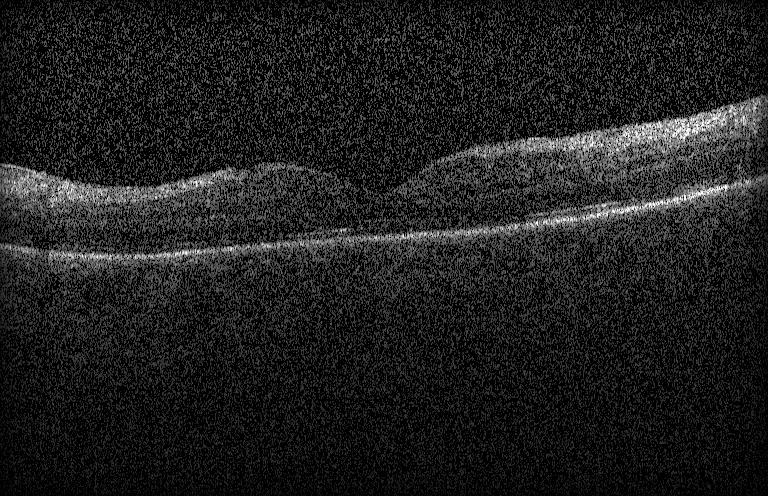

Macular scan · spectral-domain optical coherence tomography · optical coherence tomography scan. No choroidal neovascularization, no diabetic macular edema, and no drusen.